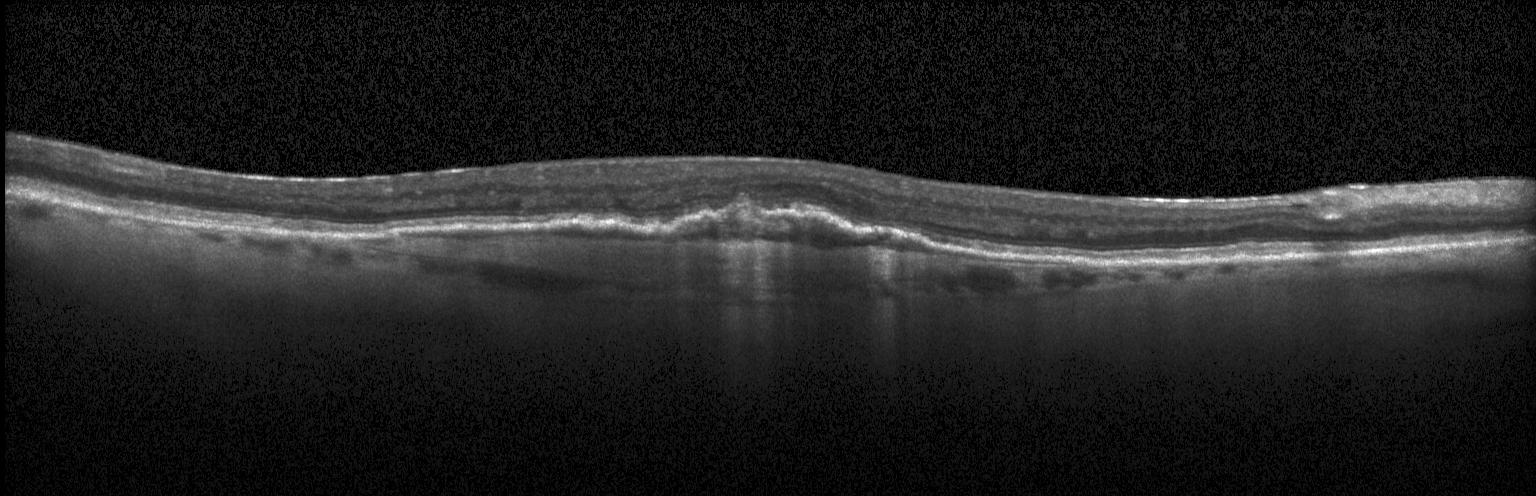
Horizontal scan through the fovea. OCT line scan. Acquired on a Heidelberg Spectralis. Spectral-domain OCT — Impression: choroidal neovascularization.